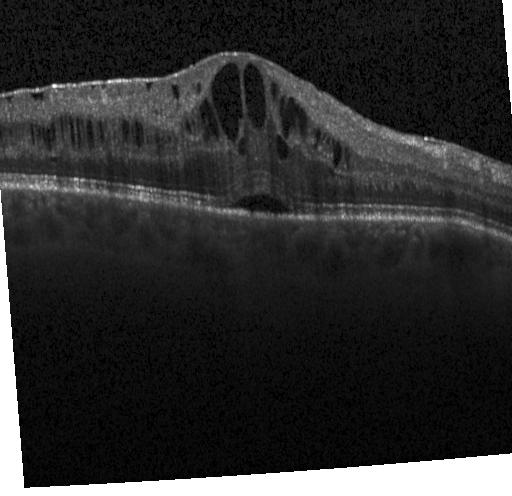

Optical coherence tomography B-scan · Heidelberg Spectralis
Finding: diabetic macular edema.